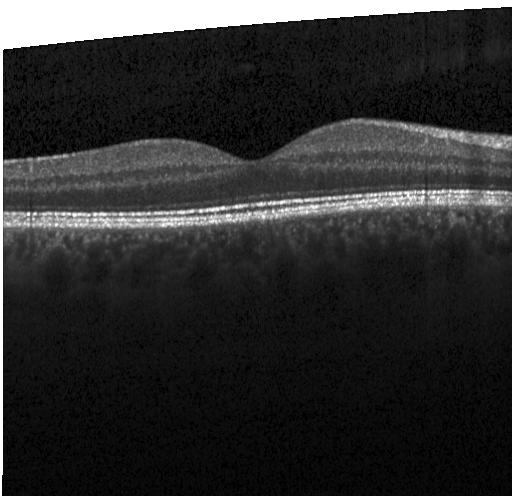 No evidence of choroidal neovascularization, diabetic macular edema, or drusen.